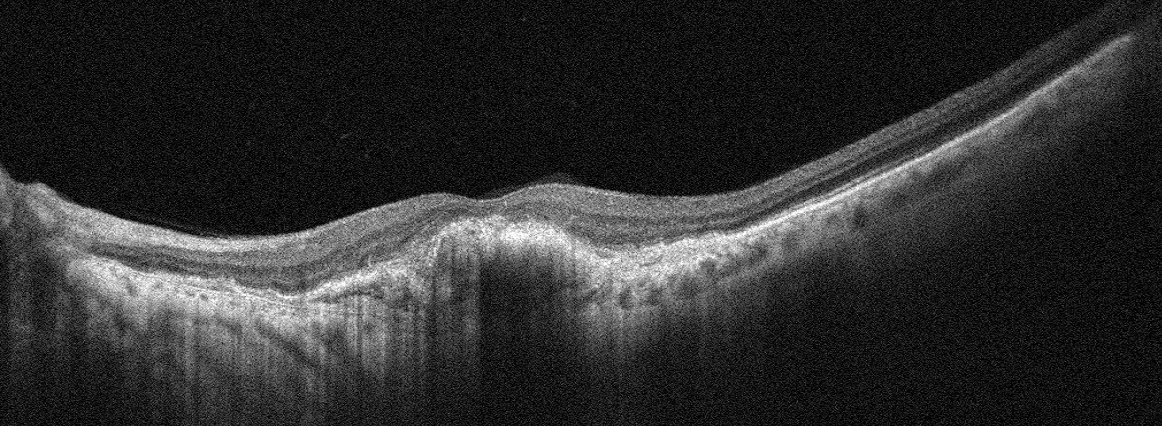
Macular scan; optical coherence tomography scan; Optovue Avanti RTVue XR; left eye.
This B-scan demonstrates AMD.